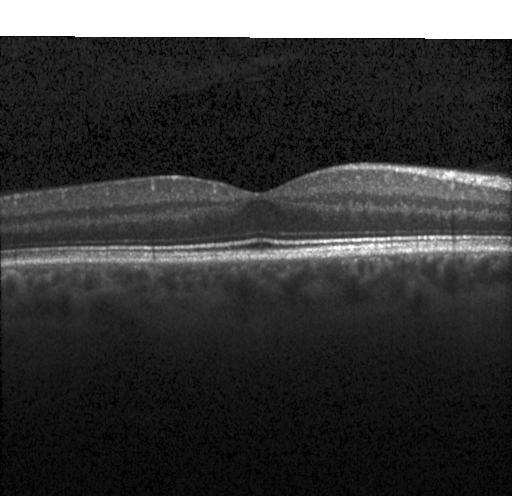 Acquired on a Heidelberg Spectralis; optical coherence tomography B-scan.
Finding: no choroidal neovascularization, diabetic macular edema, or drusen.